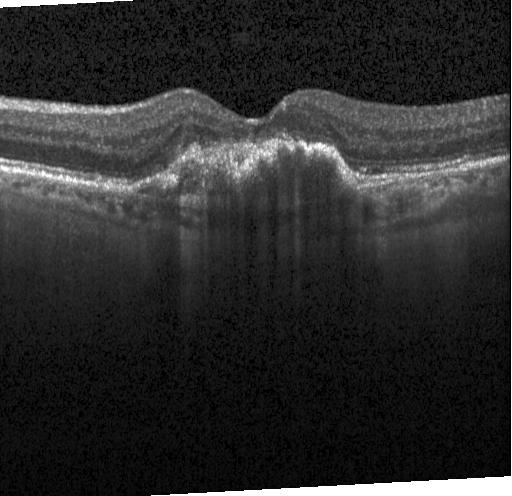 OCT line scan.
Finding: choroidal neovascularization.